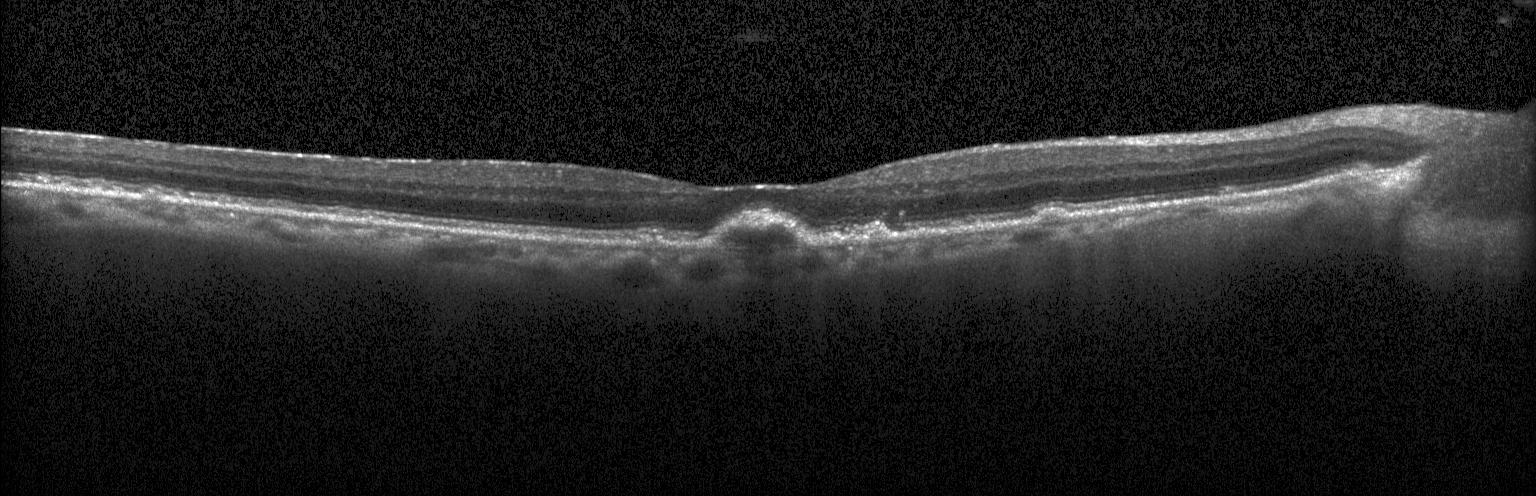

Macular scan. Acquired on a Heidelberg Spectralis. OCT B-scan
Impression: a choroidal neovascular membrane.